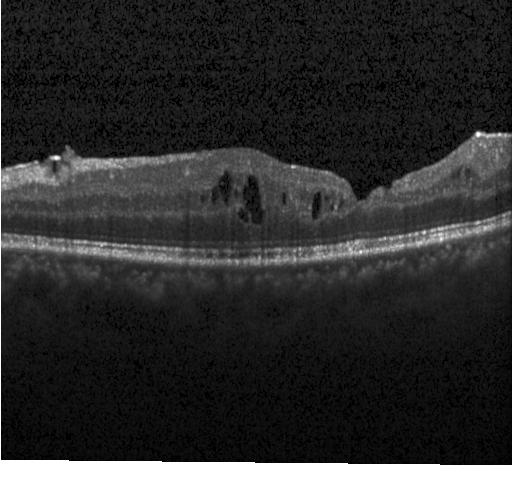 OCT B-scan, acquired on a Heidelberg Spectralis, horizontal scan through the fovea — Finding: diabetic macular edema (DME).